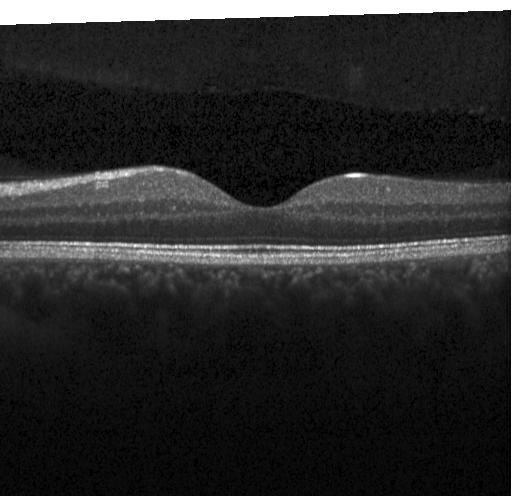
OCT line scan. Heidelberg Spectralis. SD-OCT. This B-scan demonstrates no evidence of choroidal neovascularization, diabetic macular edema, or drusen.